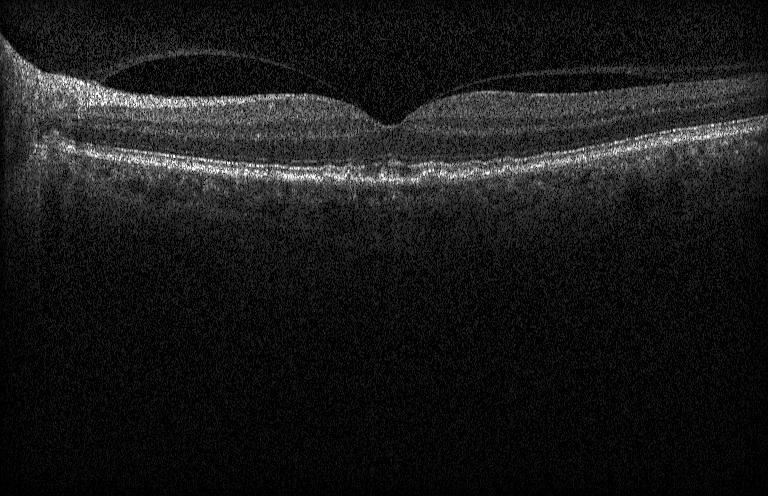
Finding: sub-RPE drusenoid deposits.